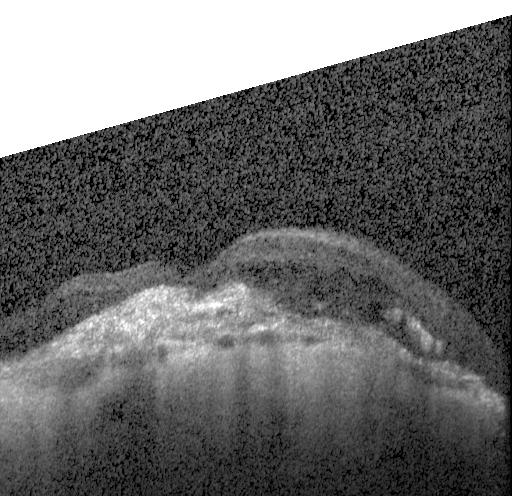

Through the macula · spectral-domain OCT · OCT B-scan · Heidelberg Spectralis OCT system. Macular OCT: choroidal neovascularization (CNV).